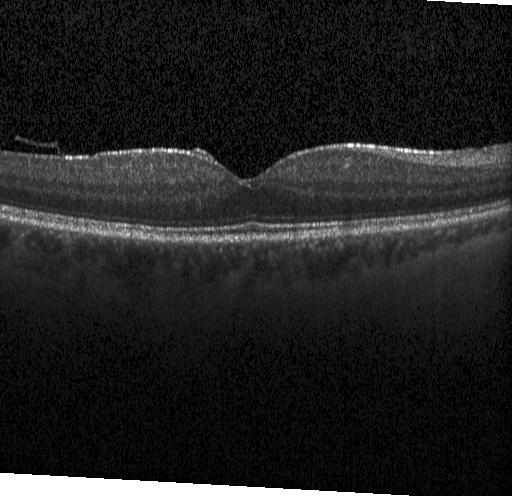

Macular scan · OCT line scan · Heidelberg Spectralis · SD-OCT
Impression: neither choroidal neovascularization, diabetic macular edema, nor drusen.